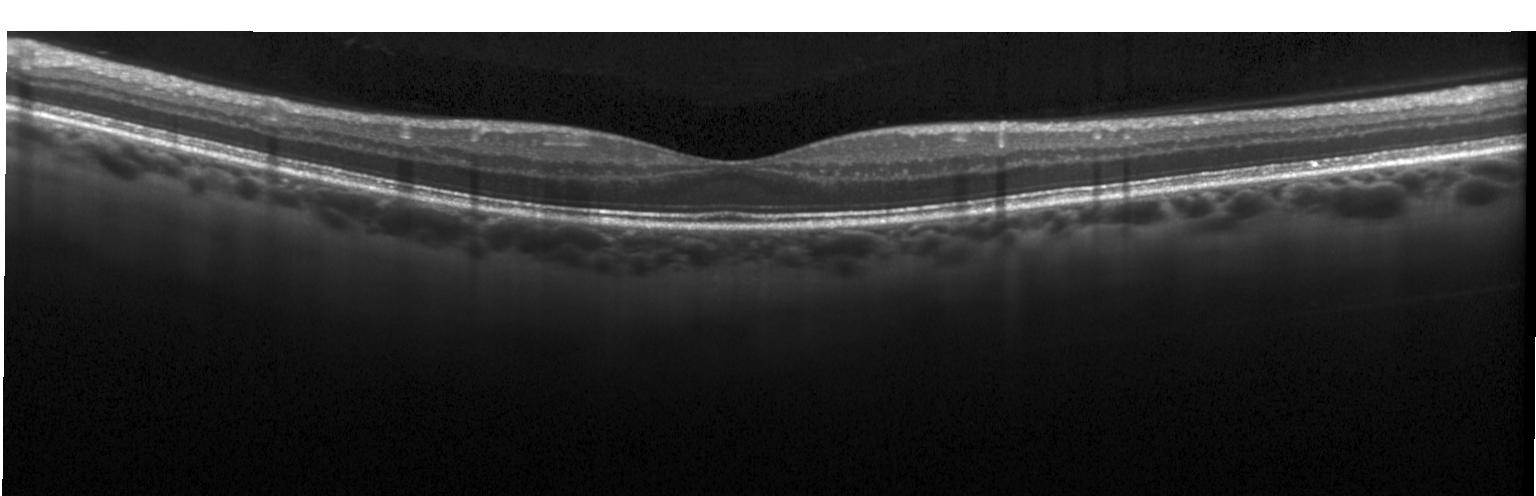 Heidelberg Spectralis; horizontal scan through the fovea; spectral-domain OCT; OCT B-scan — This B-scan demonstrates no CNV, no DME, and no drusen.